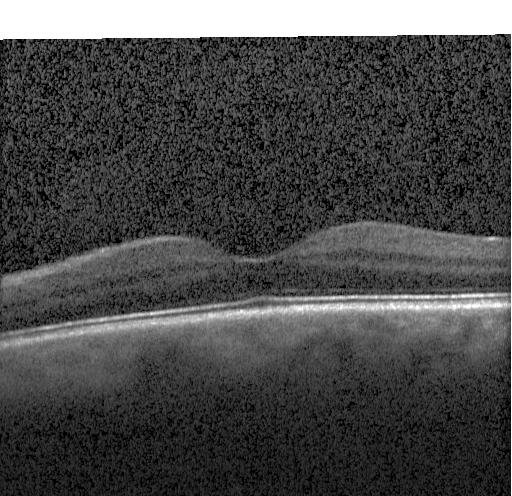 Heidelberg Spectralis OCT system; spectral-domain optical coherence tomography; optical coherence tomography B-scan
Assessment: no evidence of choroidal neovascularization, diabetic macular edema, or drusen.